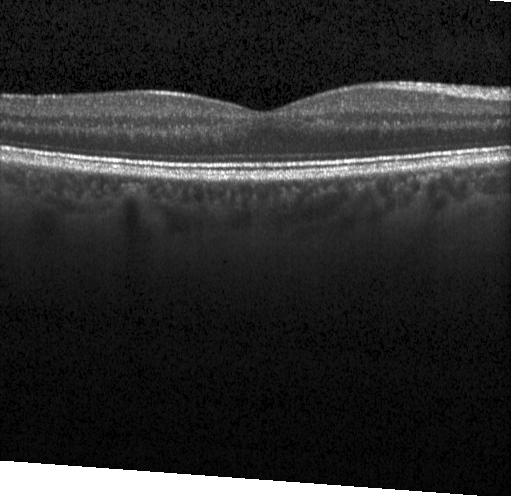
Retinal OCT cross-section
Impression: no CNV, no DME, and no drusen.